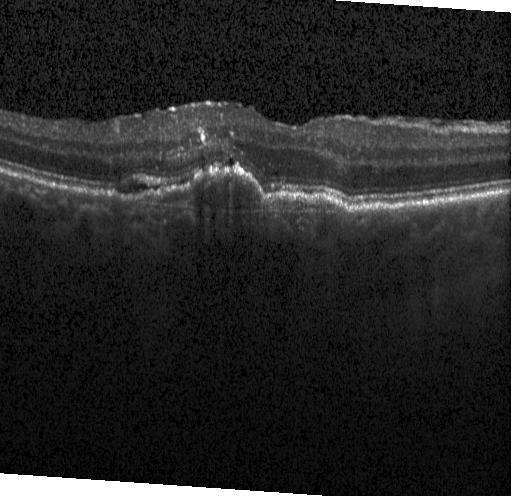 OCT line scan
OCT finding: a choroidal neovascular membrane.